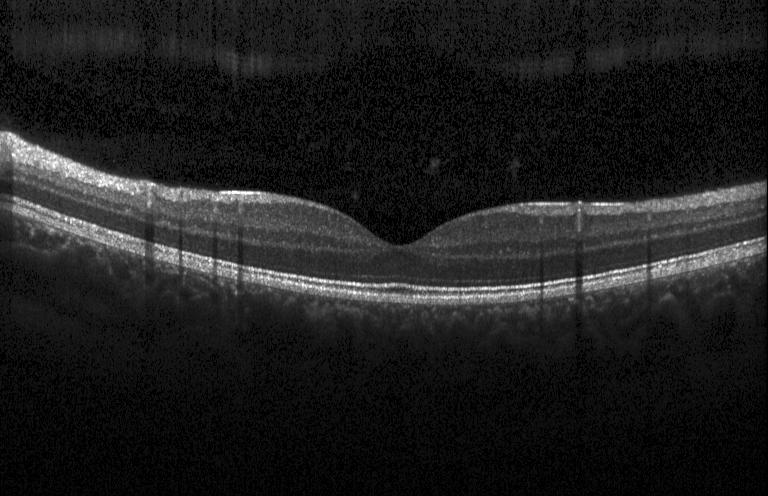
Diagnosis: no choroidal neovascularization, no diabetic macular edema, and no drusen.